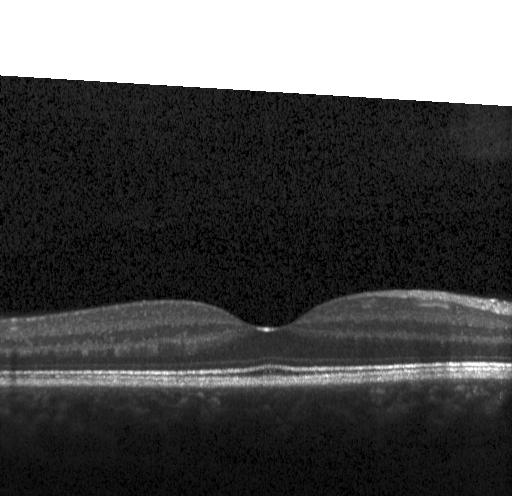
Macular OCT: no choroidal neovascularization, no diabetic macular edema, and no drusen.